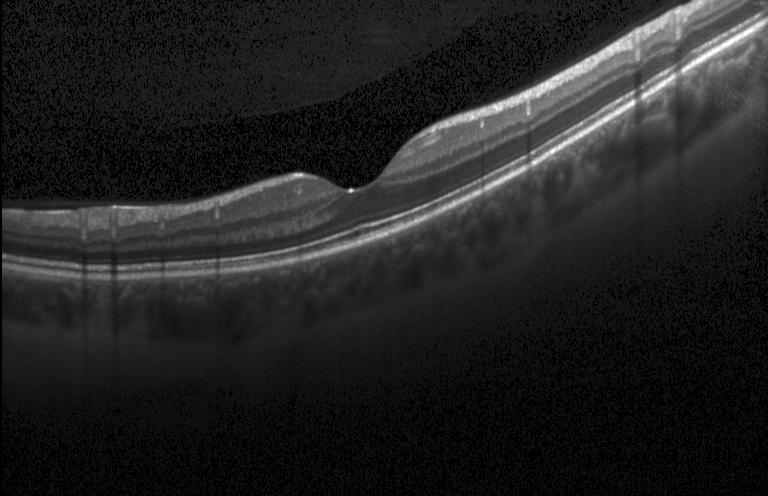
SD-OCT. Centered on the fovea. Heidelberg Spectralis. OCT B-scan — Impression: no evidence of choroidal neovascularization, diabetic macular edema, or drusen.